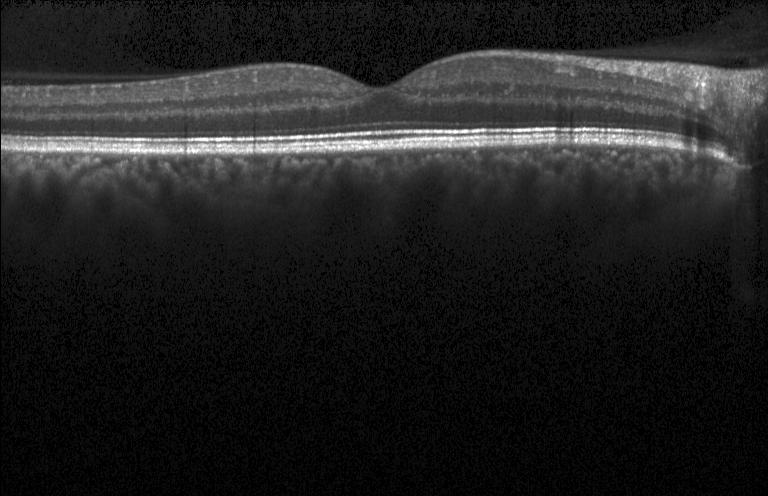 OCT line scan — Diagnosis: no evidence of choroidal neovascularization, diabetic macular edema, or drusen.